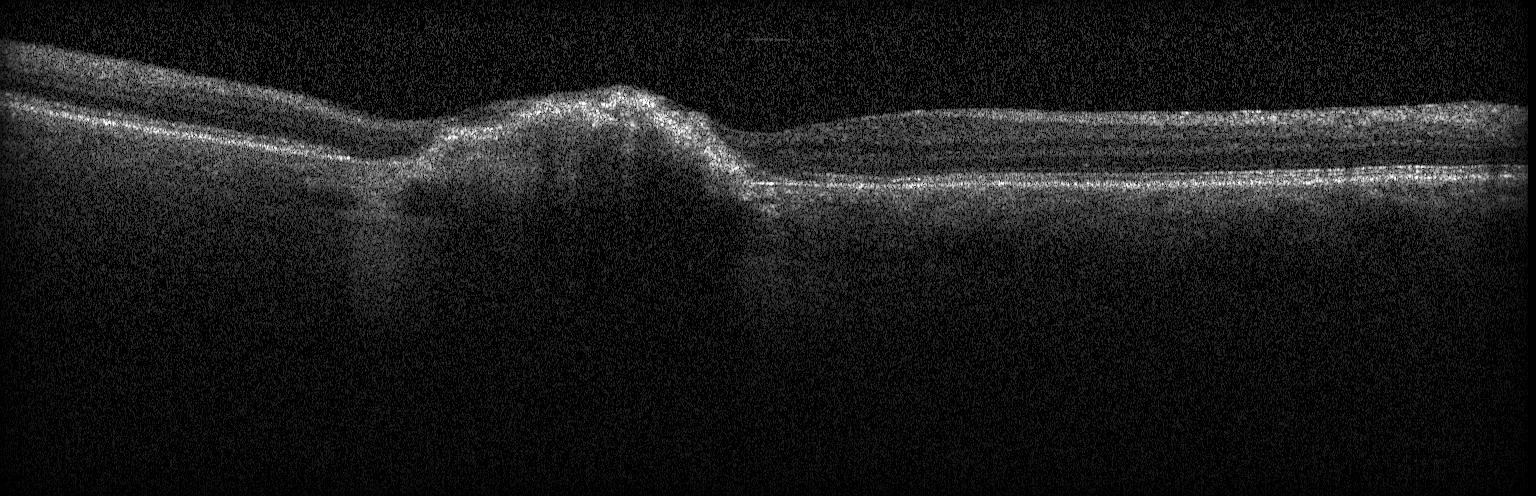
Optical coherence tomography scan · acquired on a Heidelberg Spectralis · spectral-domain OCT · macular scan.
Assessment: a choroidal neovascular membrane.